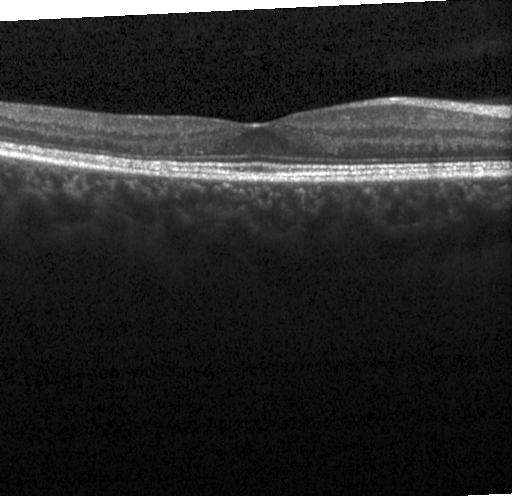

Diagnosis: no evidence of choroidal neovascularization, diabetic macular edema, or drusen.